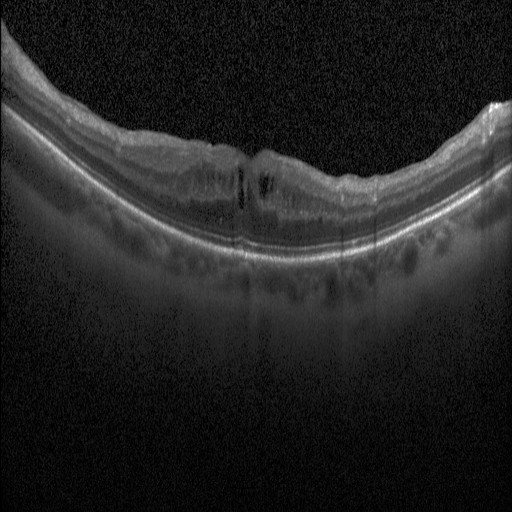

Diagnosis: DME.